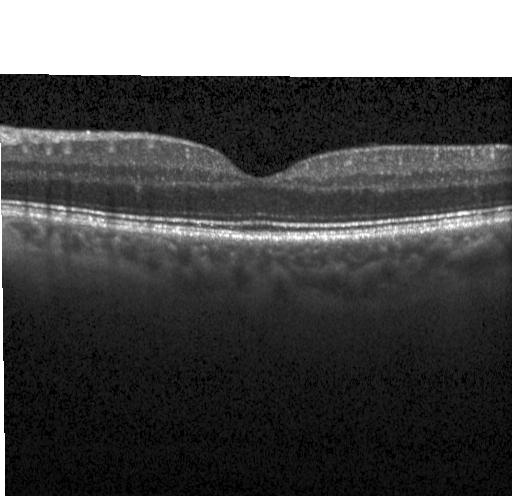

Centered on the fovea; OCT B-scan; Heidelberg Spectralis OCT system; spectral-domain OCT. OCT finding: neither CNV, DME, nor drusen.